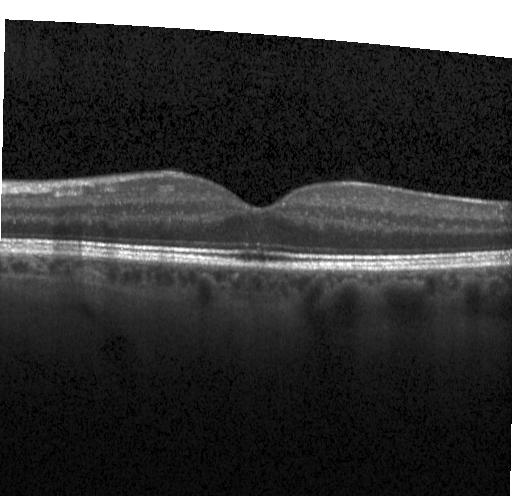
Optical coherence tomography scan; acquired on a Heidelberg Spectralis; spectral-domain optical coherence tomography; through the macula. Diagnosis: neither choroidal neovascularization, diabetic macular edema, nor drusen.